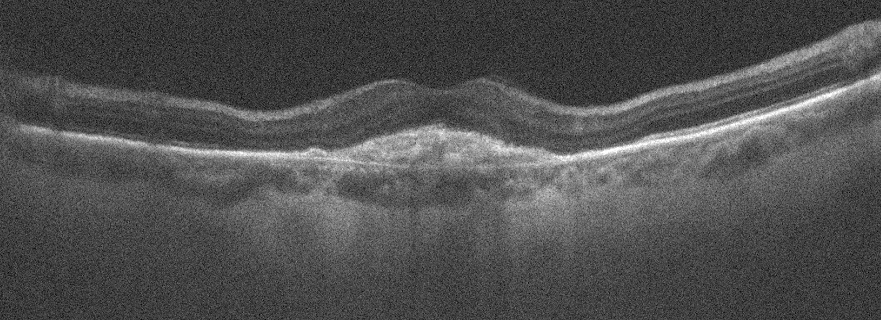
OCT B-scan; acquired on an Optovue Avanti RTVue XR.
Diagnosis: age-related macular degeneration (AMD).